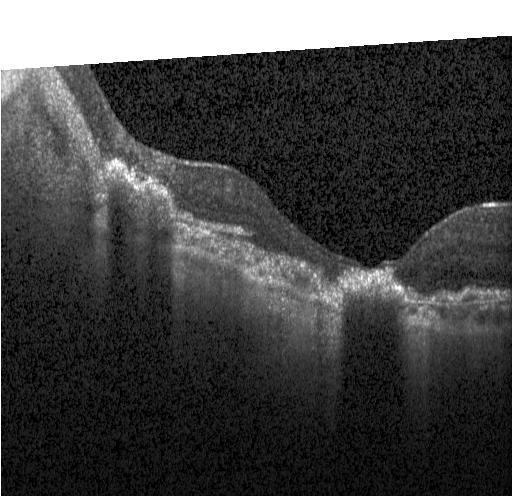 SD-OCT; OCT line scan; Heidelberg Spectralis OCT system — Macular OCT: a choroidal neovascular membrane.